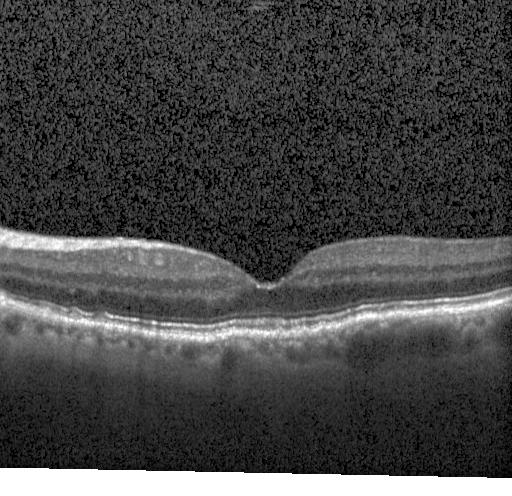

Optical coherence tomography B-scan.
Assessment: sub-RPE drusenoid deposits.